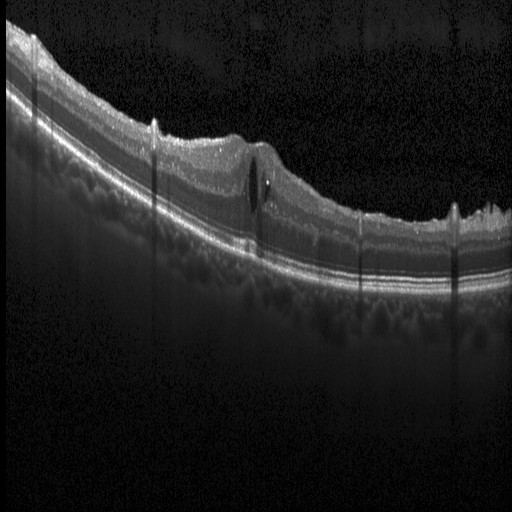
Spectral-domain OCT, horizontal scan through the fovea, retinal OCT B-scan. Macular OCT: DME.